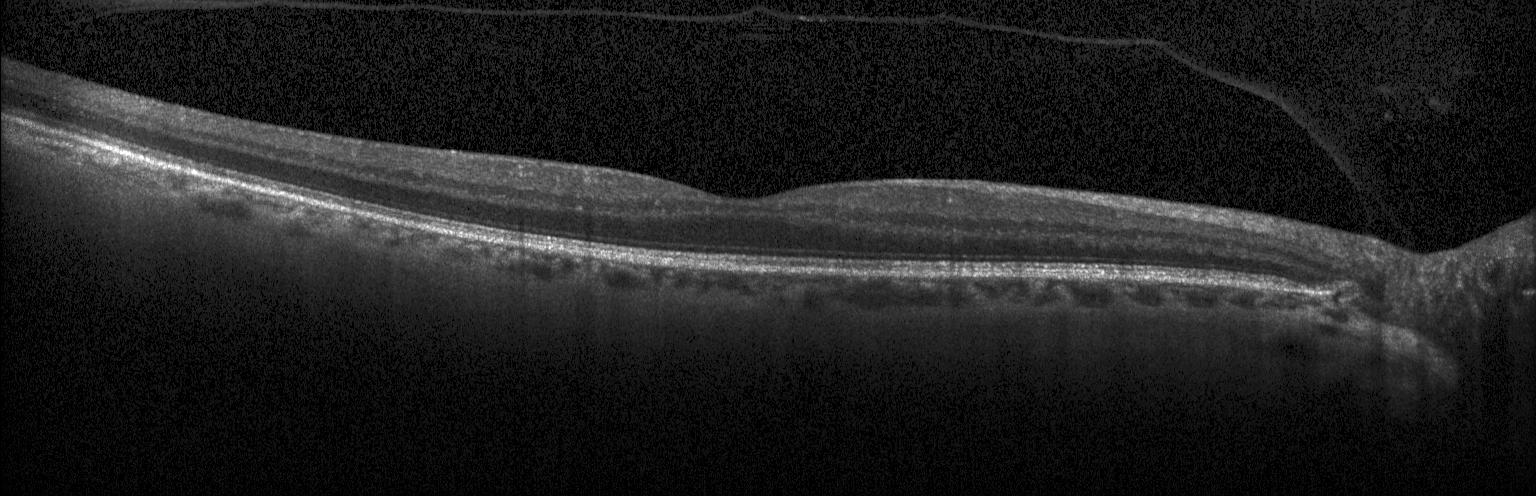 OCT line scan, fovea-centered, acquired on a Heidelberg Spectralis, SD-OCT. Diagnosis: no choroidal neovascularization, diabetic macular edema, or drusen.